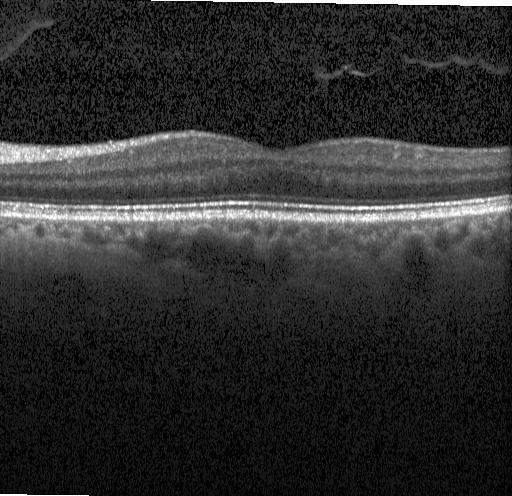
Heidelberg Spectralis. Through the macula. Optical coherence tomography scan
Impression: neither choroidal neovascularization, diabetic macular edema, nor drusen.